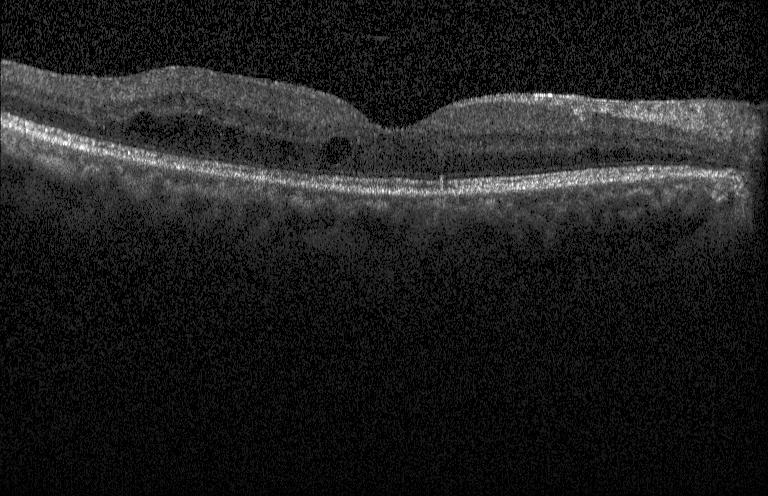
Retinal OCT cross-section showing DME.